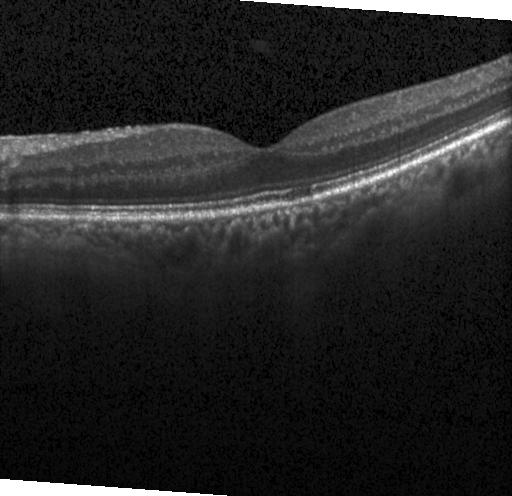 Optical coherence tomography scan — Diagnosis: no CNV, no DME, and no drusen.